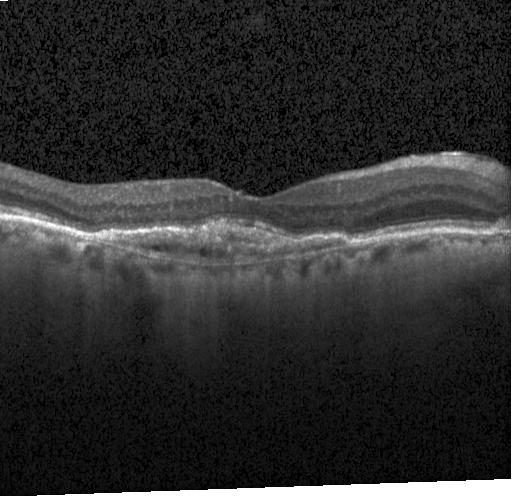 Spectral-domain OCT, retinal OCT cross-section — The scan shows choroidal neovascularization.